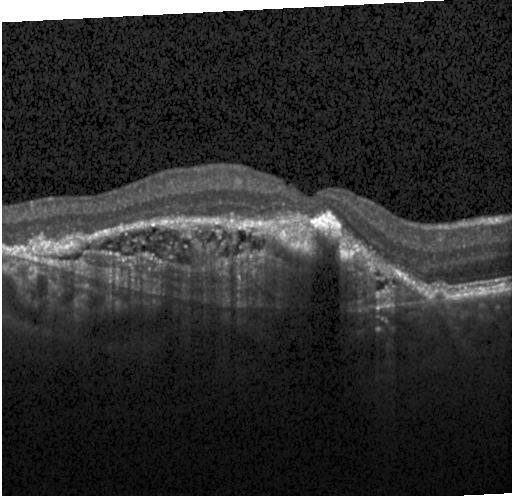

This B-scan demonstrates choroidal neovascularization (CNV).